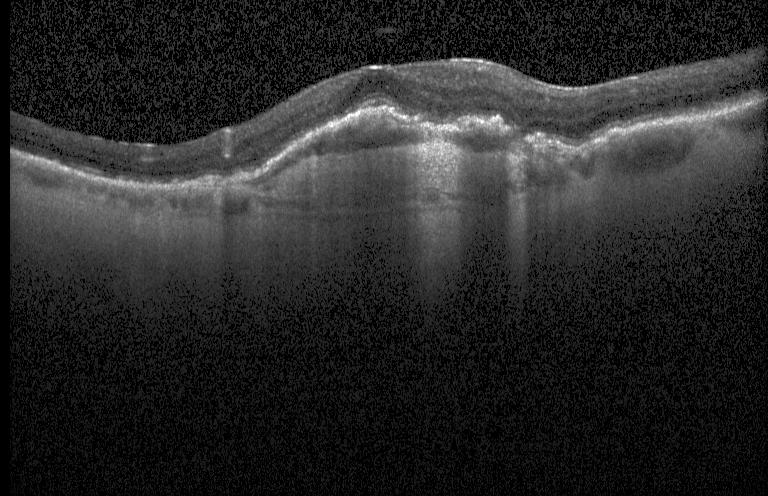 Finding: CNV.